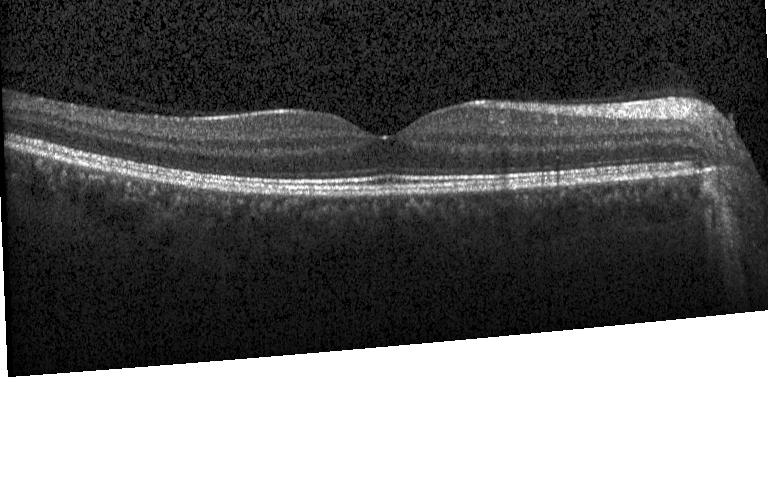
Diagnosis: no choroidal neovascularization, diabetic macular edema, or drusen.